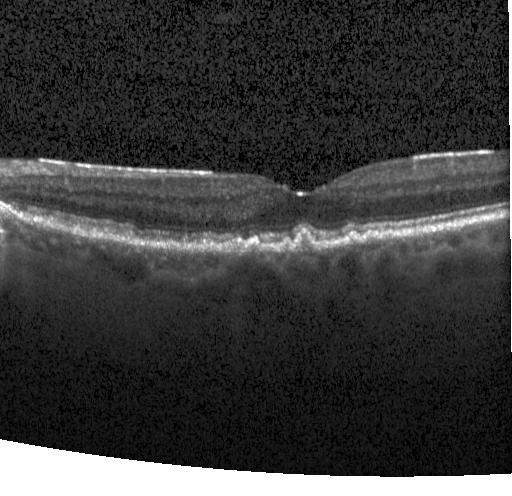
Impression: drusen.